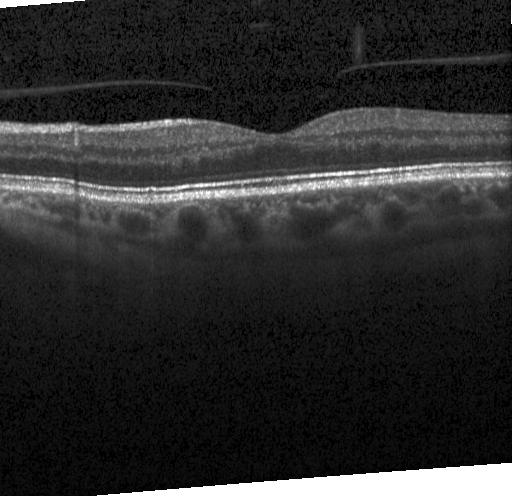 OCT B-scan showing no evidence of CNV, DME, or drusen.